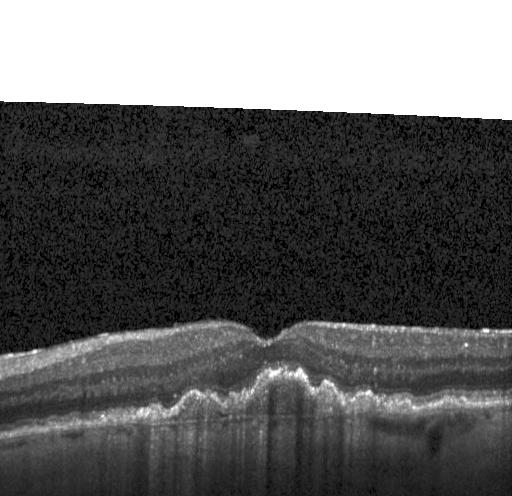

Diagnosis: a choroidal neovascular membrane.